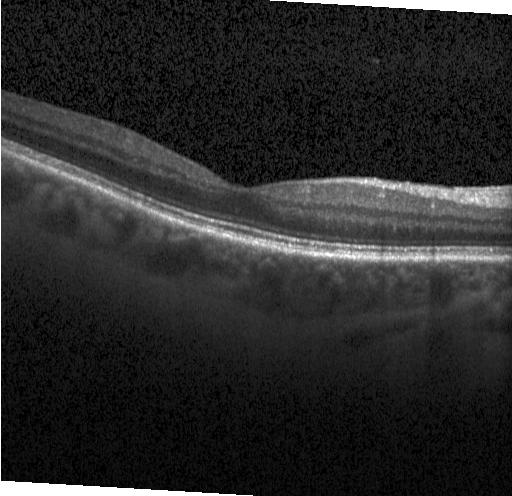
OCT B-scan. Spectral-domain optical coherence tomography. Macular scan
Dx: no evidence of choroidal neovascularization, diabetic macular edema, or drusen.